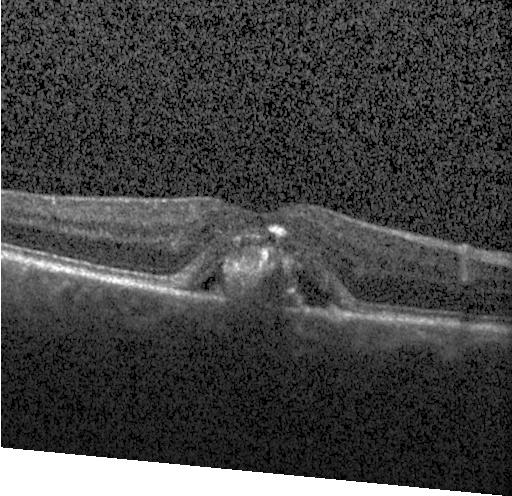
Impression: a choroidal neovascular membrane.